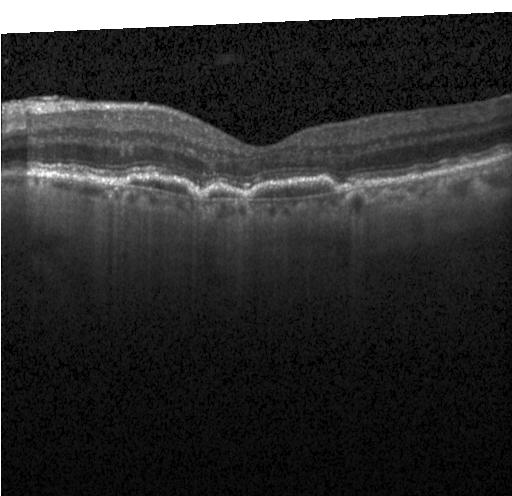

Diagnosis: CNV.